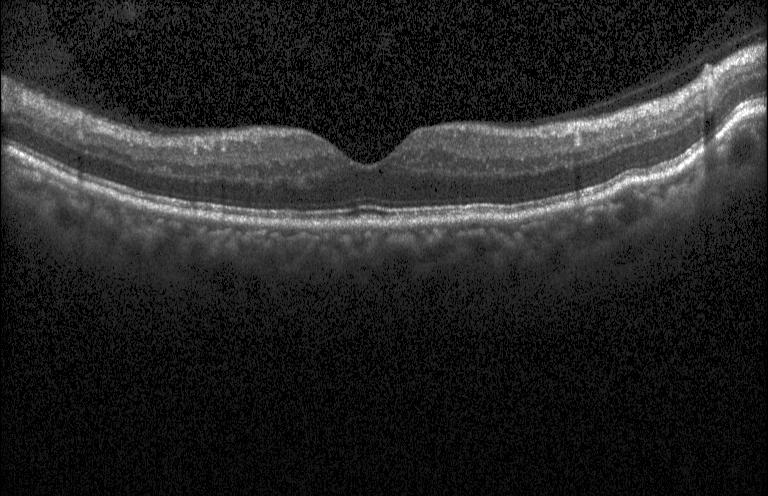

Diagnosis: neither CNV, DME, nor drusen.